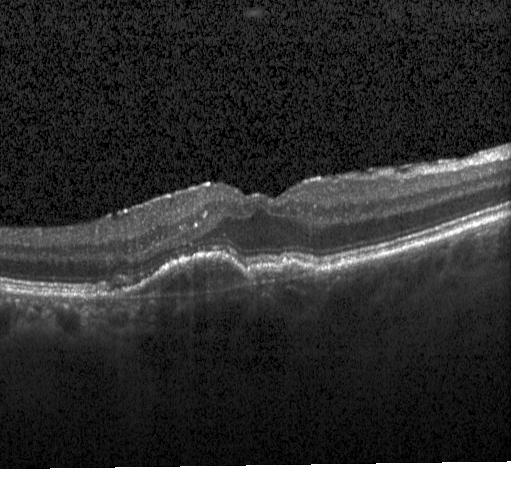
OCT finding: a choroidal neovascular membrane.